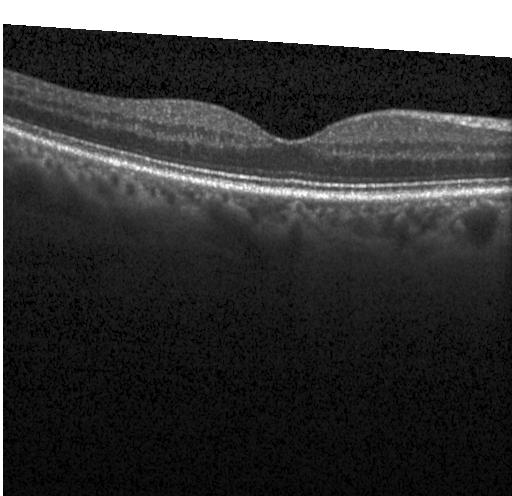

Assessment: neither choroidal neovascularization, diabetic macular edema, nor drusen.